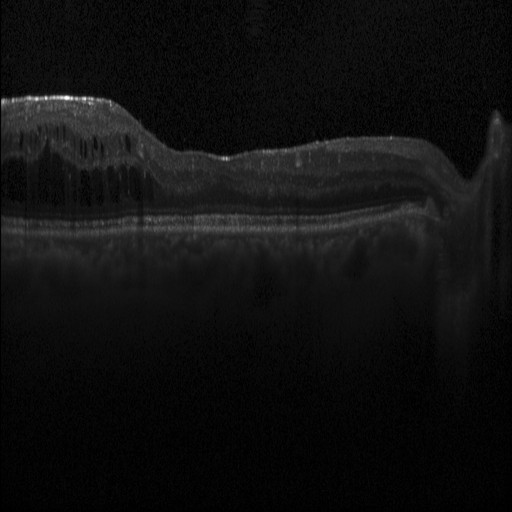
Diagnosis: DME.